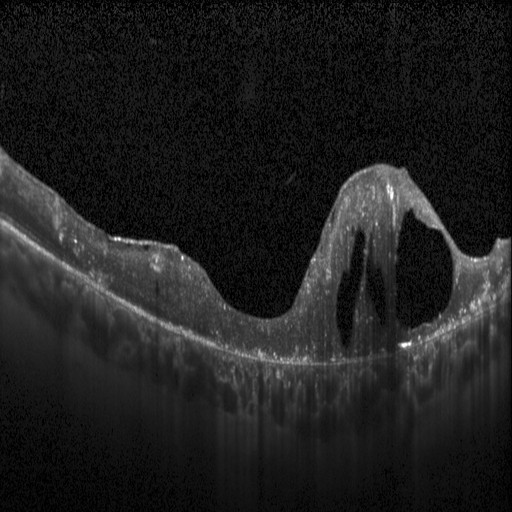 Retinal OCT B-scan
Finding: DME.